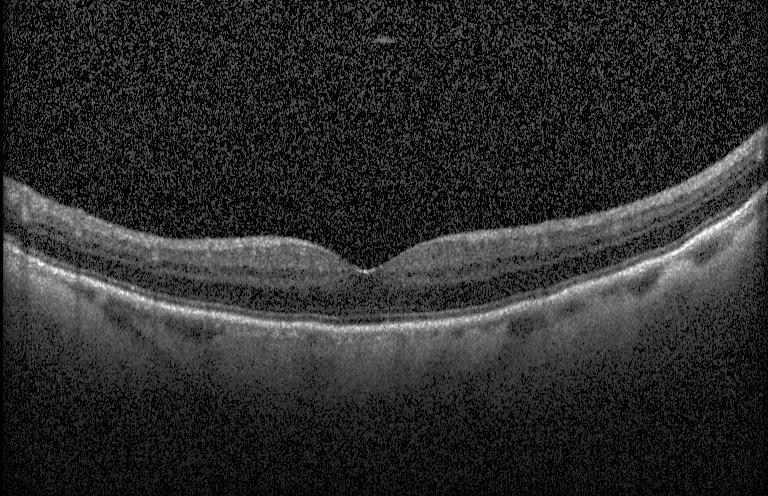
Assessment: neither choroidal neovascularization, diabetic macular edema, nor drusen.